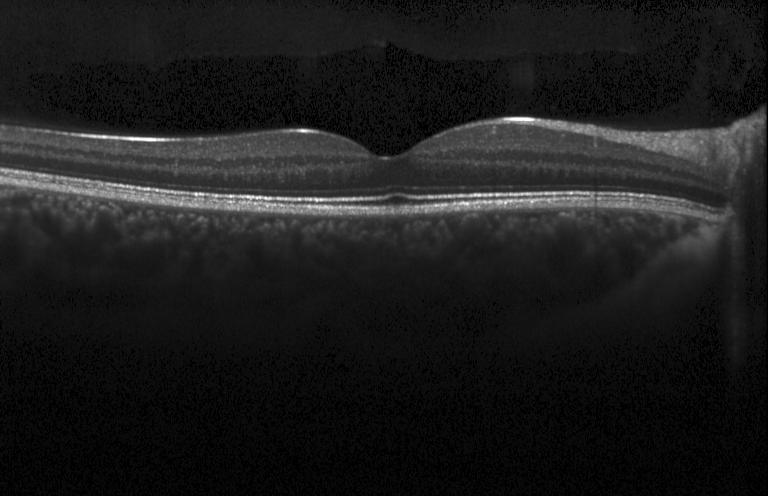

OCT line scan
Neither CNV, DME, nor drusen.